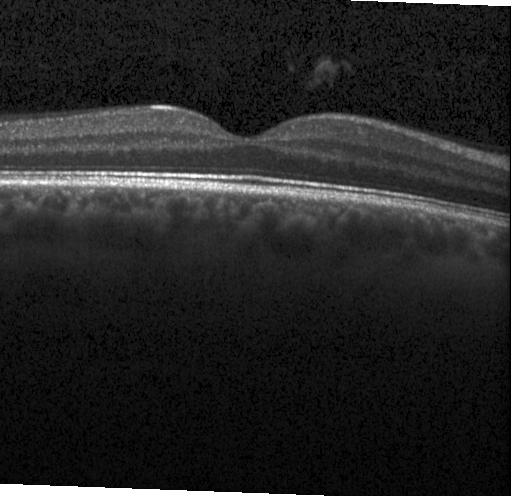 OCT line scan. Impression: no choroidal neovascularization, diabetic macular edema, or drusen.